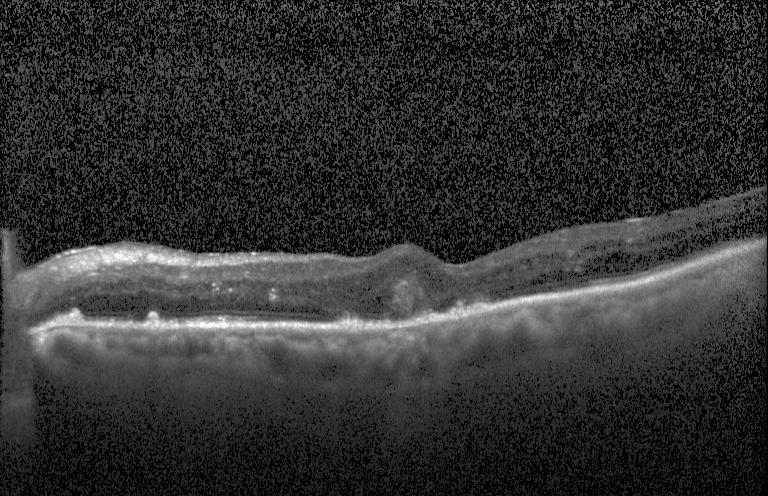 Finding: a choroidal neovascular membrane.